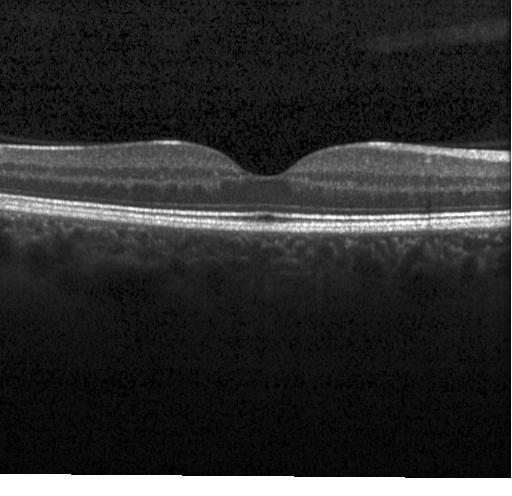

Retinal OCT cross-section, through the macula — Finding: neither CNV, DME, nor drusen.